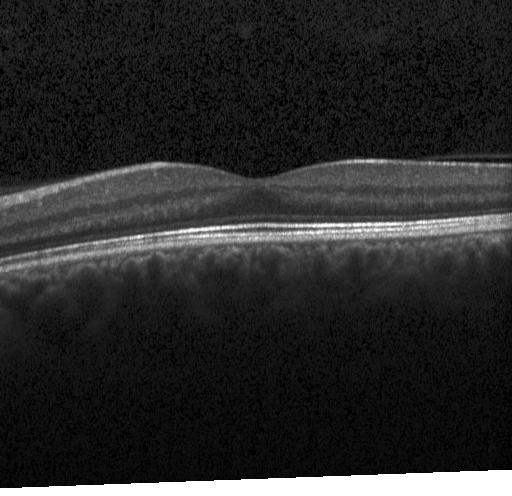

Spectral-domain optical coherence tomography; retinal OCT cross-section; horizontal scan through the fovea.
This B-scan demonstrates neither choroidal neovascularization, diabetic macular edema, nor drusen.